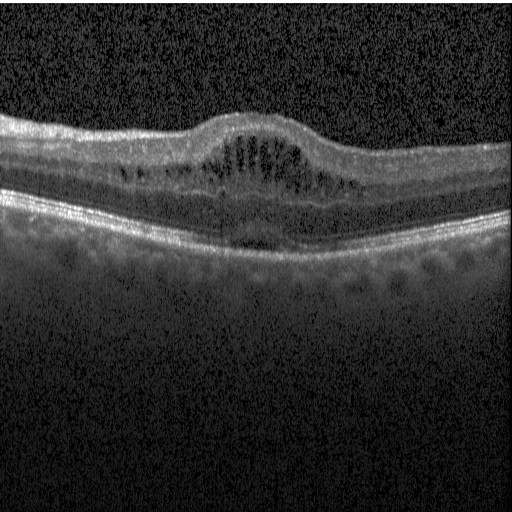

Macular OCT demonstrating DME.